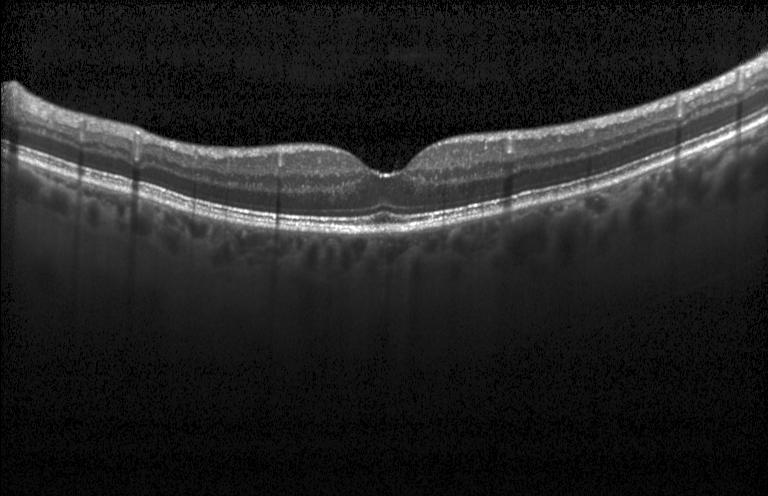
OCT scan showing neither choroidal neovascularization, diabetic macular edema, nor drusen.